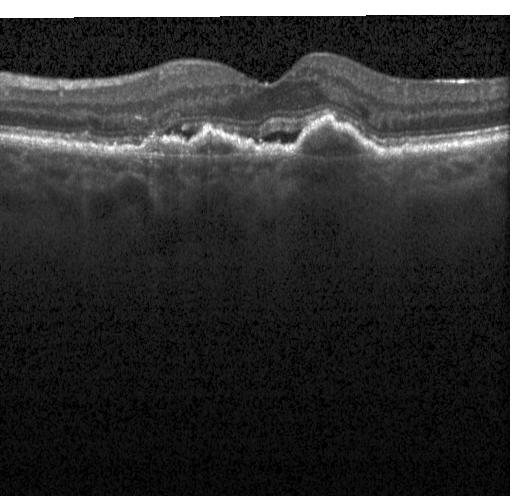
Fovea-centered · spectral-domain optical coherence tomography · Heidelberg Spectralis OCT system · optical coherence tomography B-scan
The scan shows a choroidal neovascular membrane.